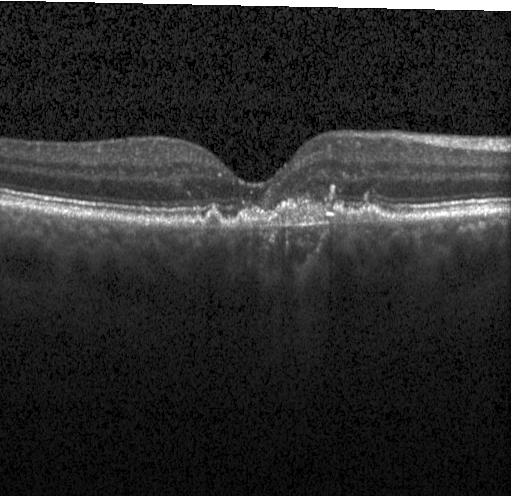

Impression: CNV.